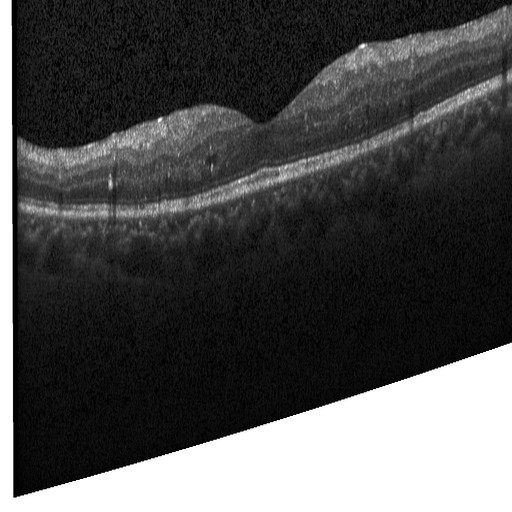 Optical coherence tomography B-scan.
Finding: DME.